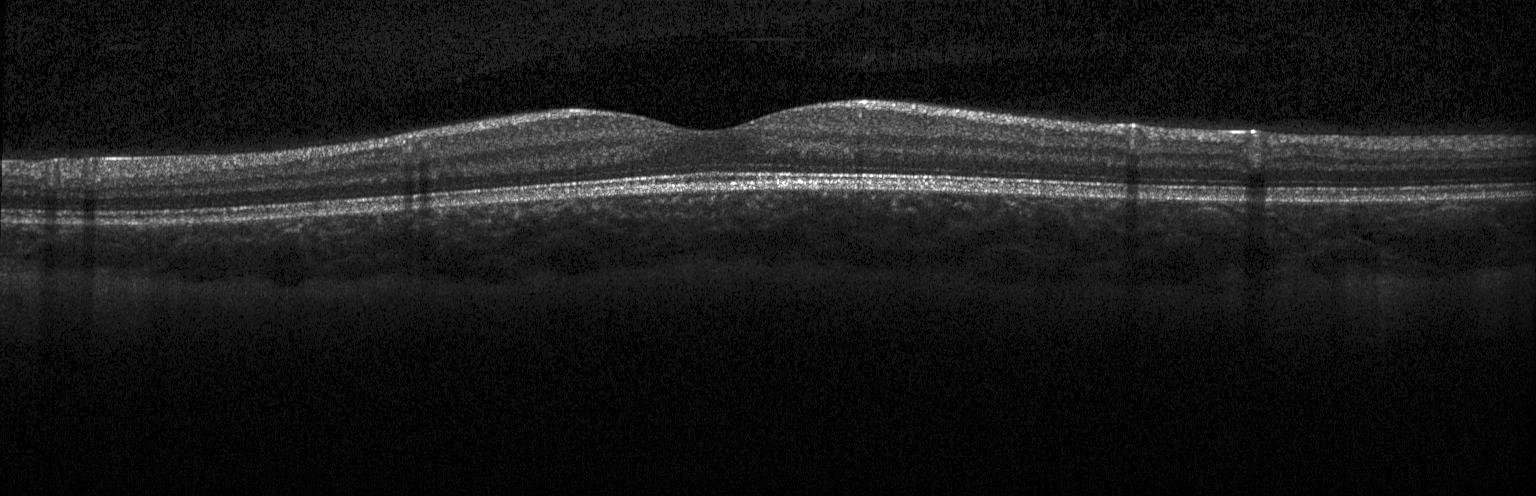
Acquired on a Heidelberg Spectralis. SD-OCT. Retinal OCT cross-section — The scan shows no choroidal neovascularization, no diabetic macular edema, and no drusen.